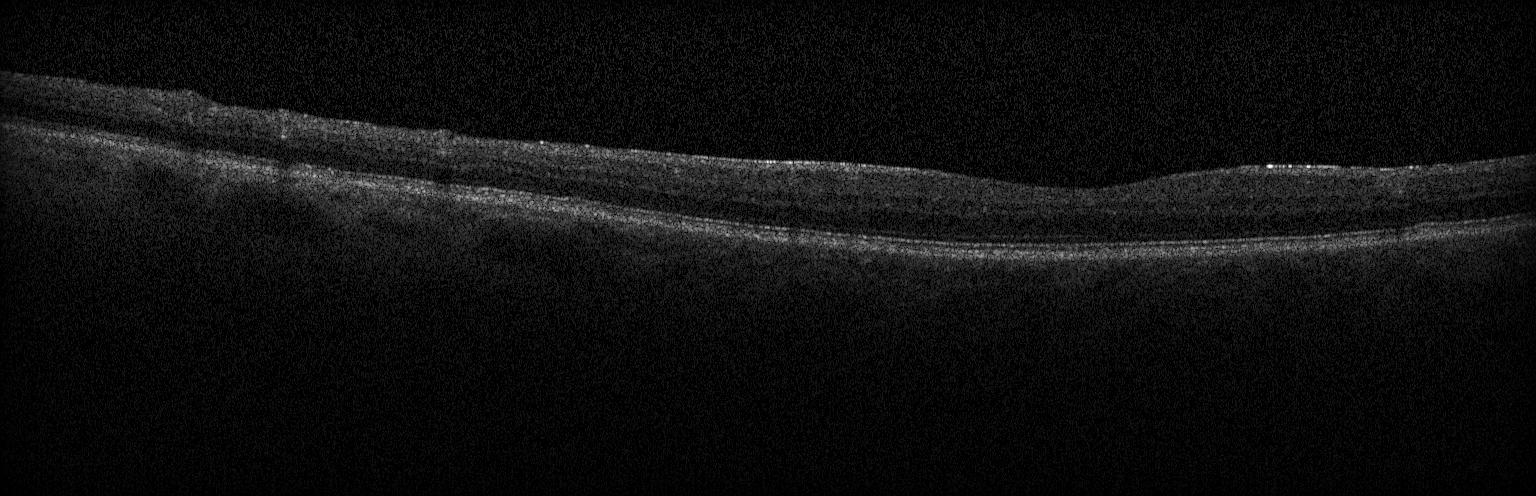 SD-OCT. Horizontal scan through the fovea. OCT line scan
Macular OCT: neither choroidal neovascularization, diabetic macular edema, nor drusen.